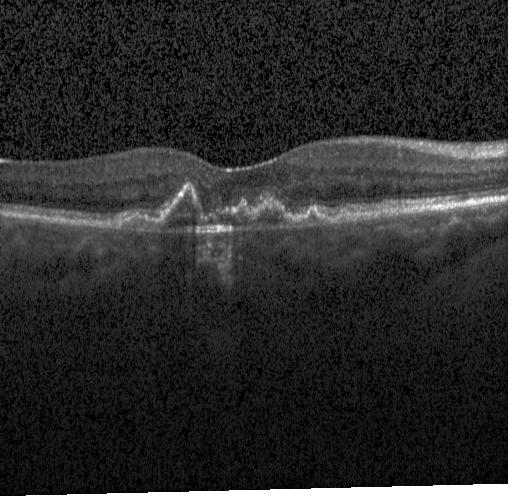

OCT finding: CNV.